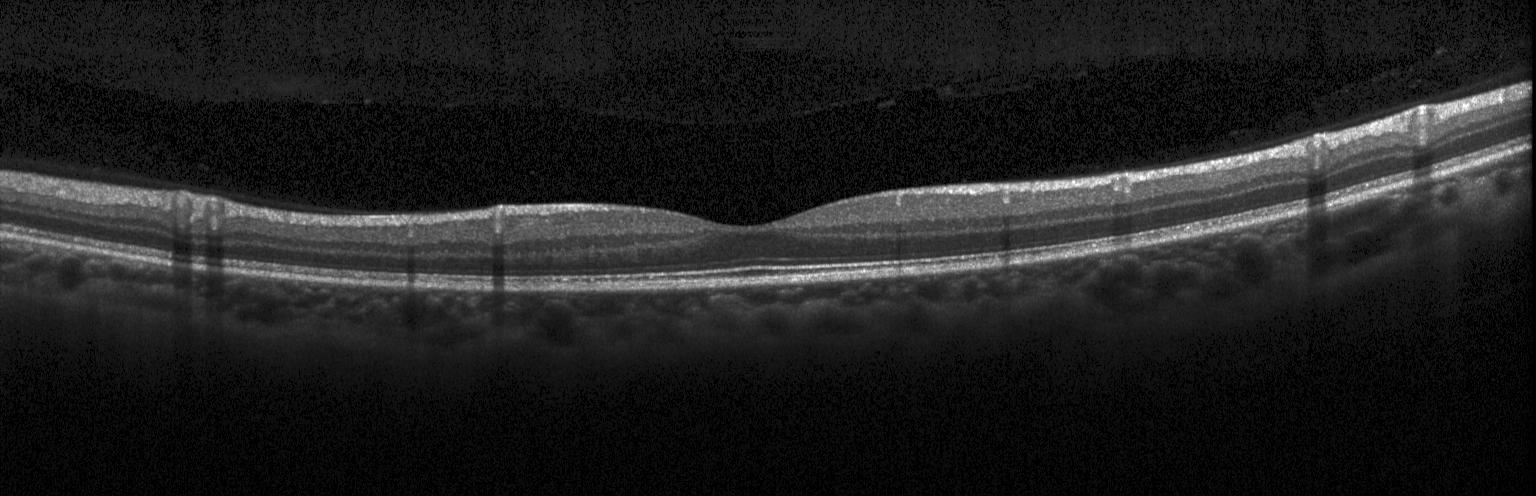
Instrument: Heidelberg Spectralis; retinal OCT cross-section; spectral-domain OCT.
Finding: no choroidal neovascularization, diabetic macular edema, or drusen.